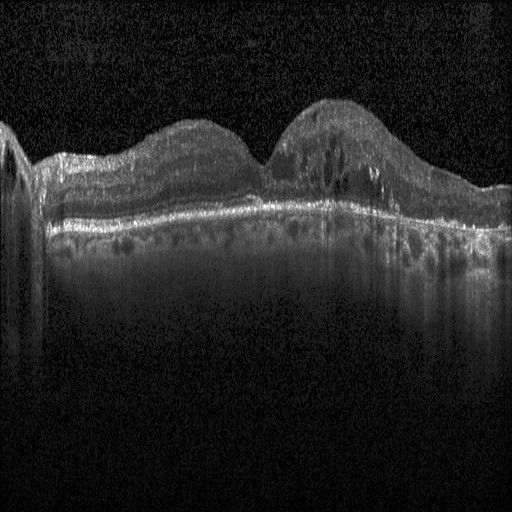 Heidelberg Spectralis. Spectral-domain optical coherence tomography. Retinal OCT cross-section. Centered on the fovea
The scan shows diabetic macular edema.